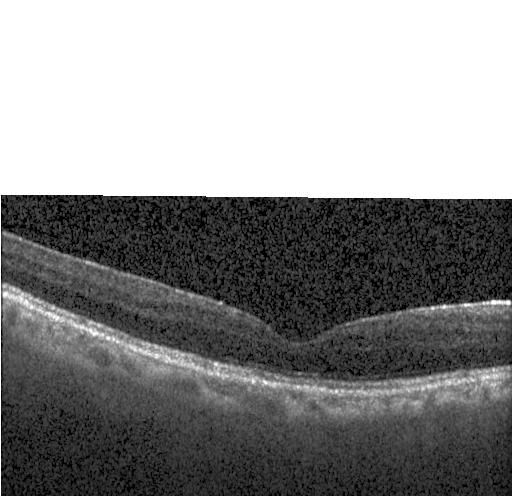 OCT B-scan showing no CNV, no DME, and no drusen.